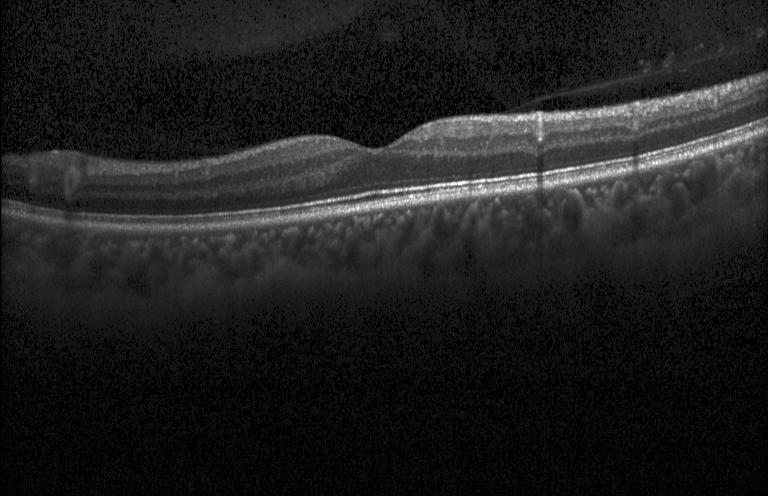
Spectral-domain OCT. Instrument: Heidelberg Spectralis. Horizontal scan through the fovea. Optical coherence tomography B-scan.
Impression: no evidence of CNV, DME, or drusen.